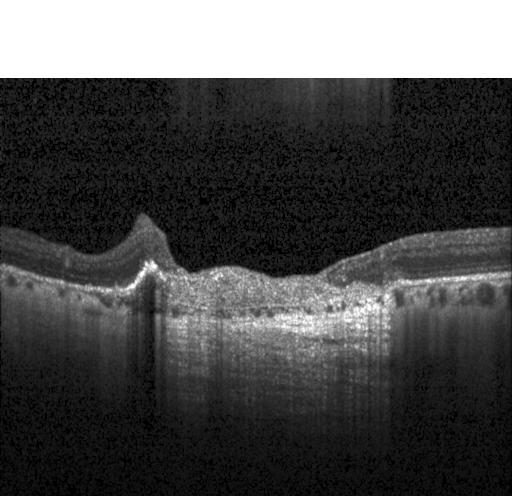
Centered on the fovea · retinal OCT cross-section · spectral-domain optical coherence tomography
OCT finding: a choroidal neovascular membrane.